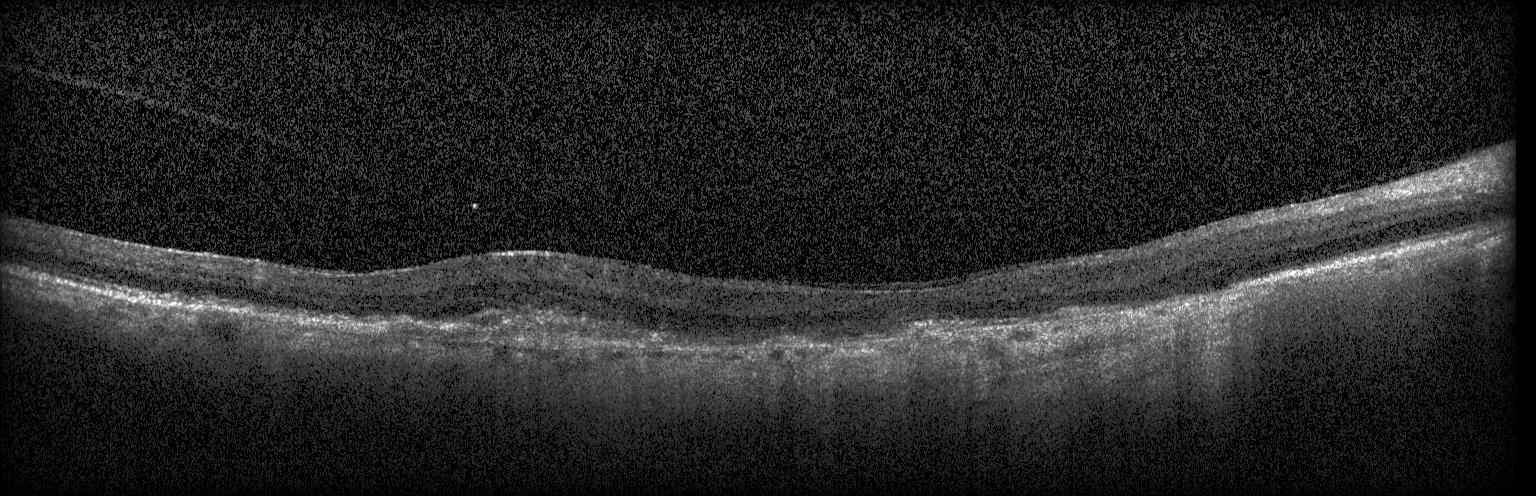

Impression: a choroidal neovascular membrane.